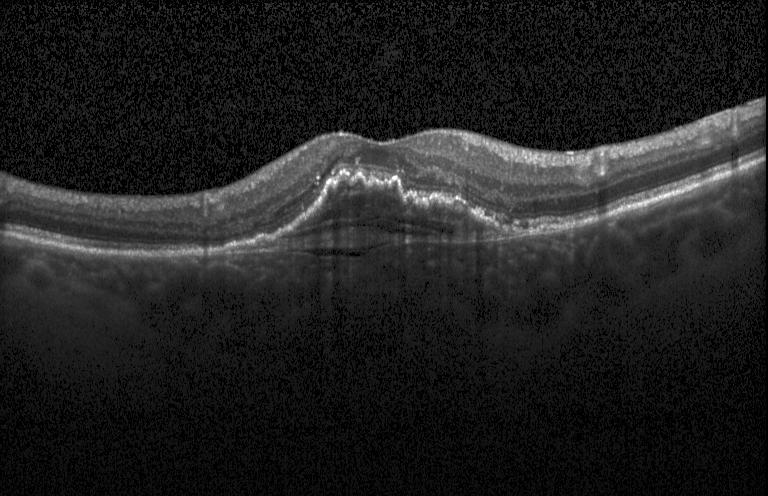
Retinal OCT cross-section showing choroidal neovascularization (CNV).